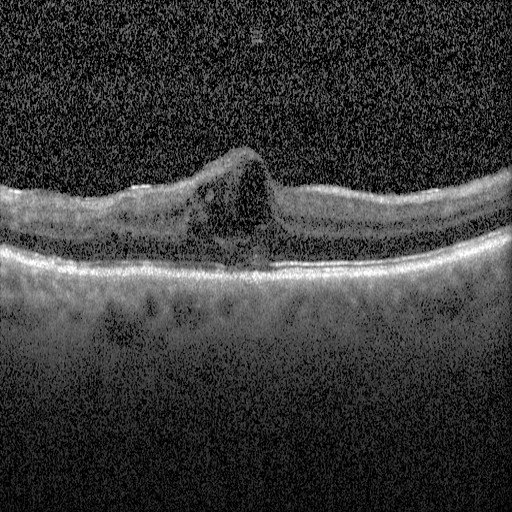 Finding: diabetic macular edema (DME).